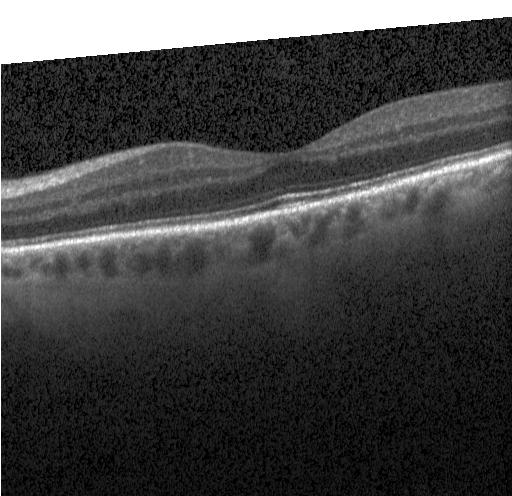
Fovea-centered, optical coherence tomography B-scan, instrument: Heidelberg Spectralis, spectral-domain OCT. Diagnosis: neither choroidal neovascularization, diabetic macular edema, nor drusen.